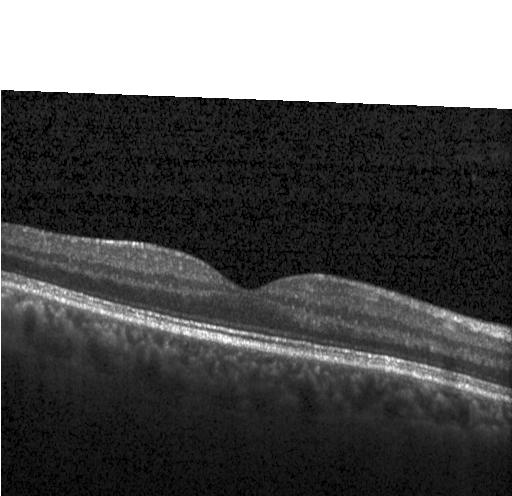 Macular OCT demonstrating no CNV, DME, or drusen.